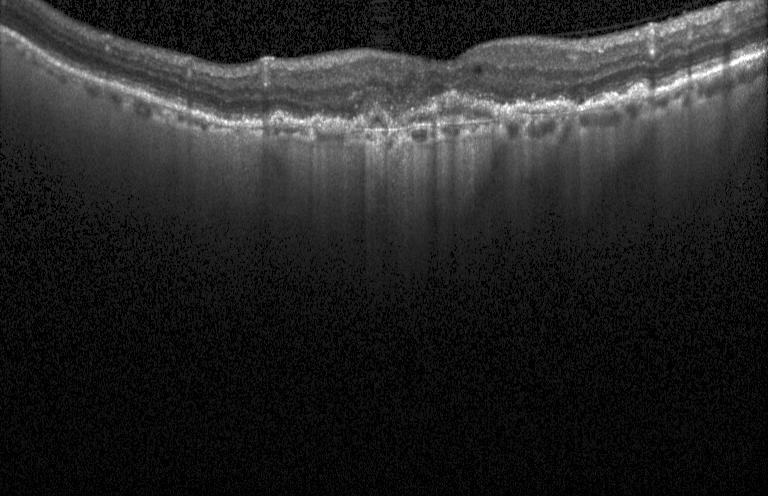

Retinal OCT B-scan
Assessment: choroidal neovascularization.